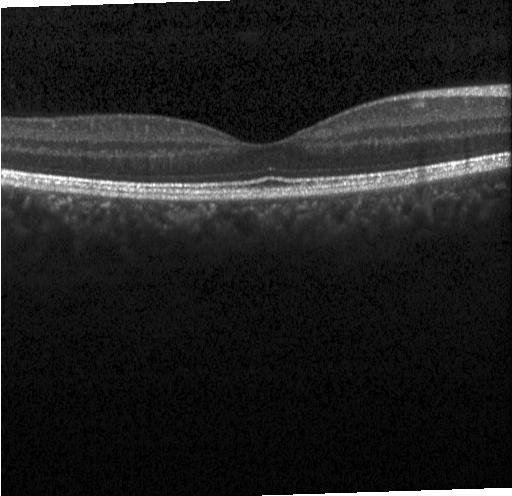
Macular OCT demonstrating no choroidal neovascularization, no diabetic macular edema, and no drusen.